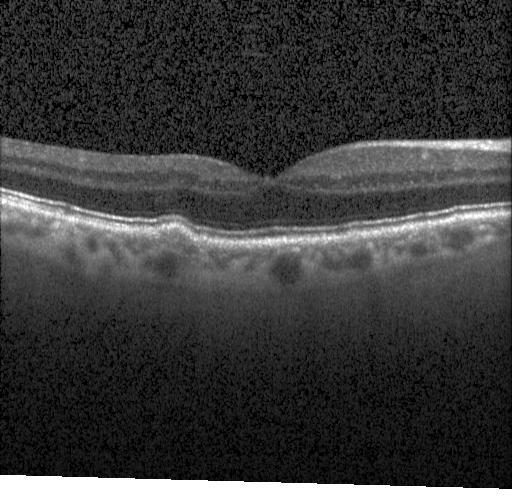
Instrument: Heidelberg Spectralis, retinal OCT B-scan.
The scan shows drusen.